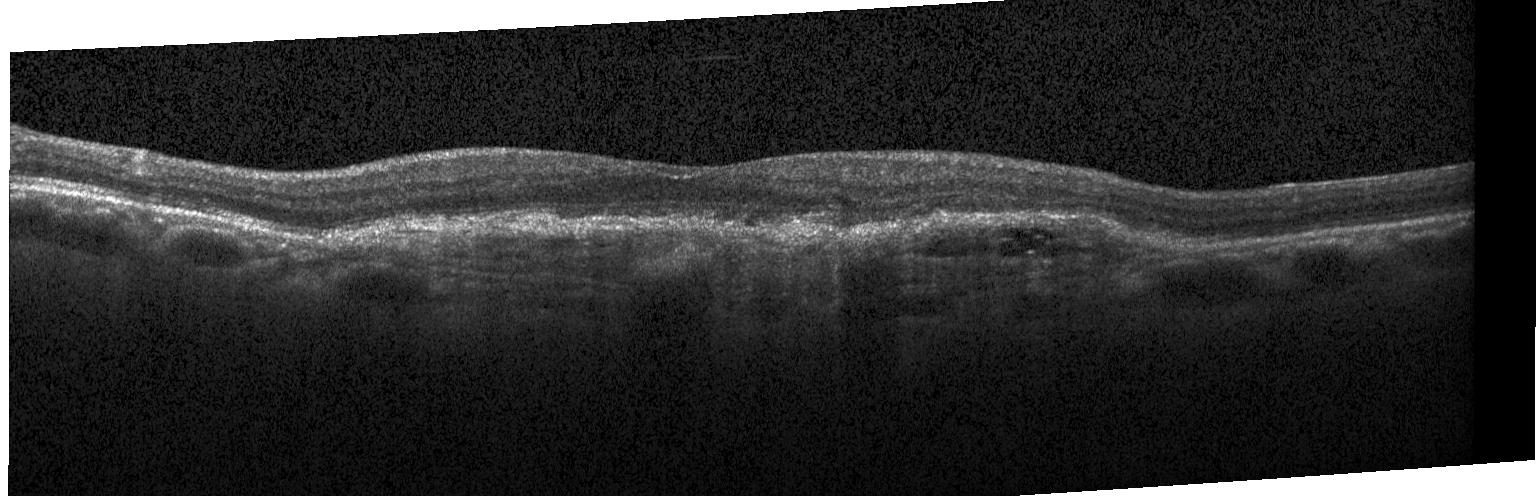
Macular scan, retinal OCT B-scan
Impression: a choroidal neovascular membrane.